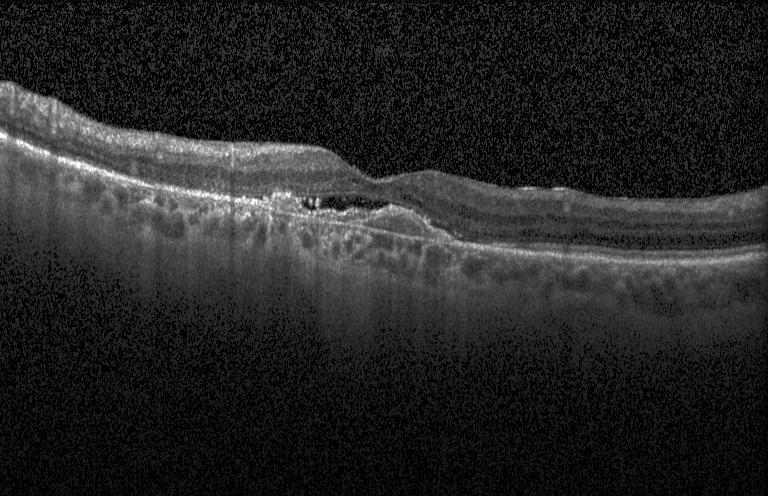 OCT finding: a choroidal neovascular membrane.